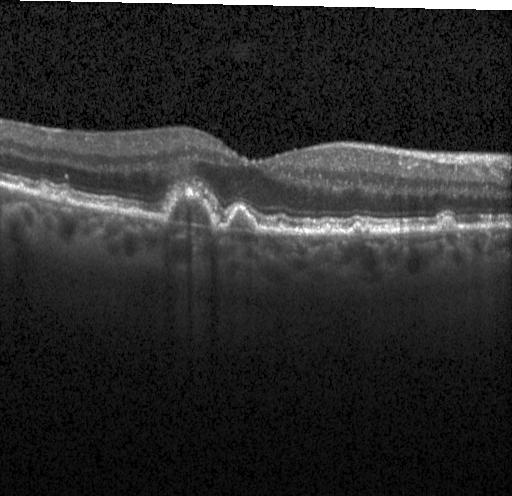 OCT line scan. Diagnosis: multiple drusen.